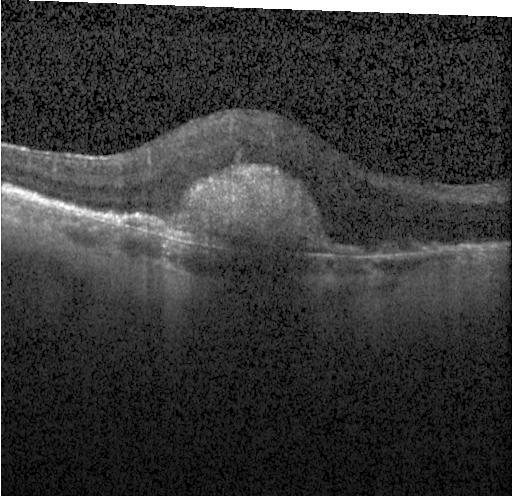
Spectral-domain optical coherence tomography · Heidelberg Spectralis · OCT line scan
The scan shows CNV.